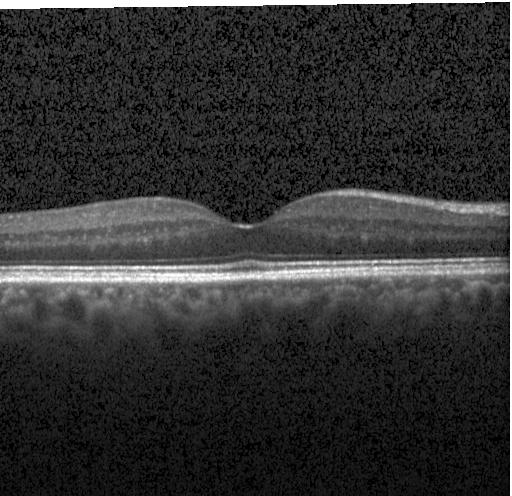
Fovea-centered. Heidelberg Spectralis. OCT line scan.
The scan shows neither choroidal neovascularization, diabetic macular edema, nor drusen.